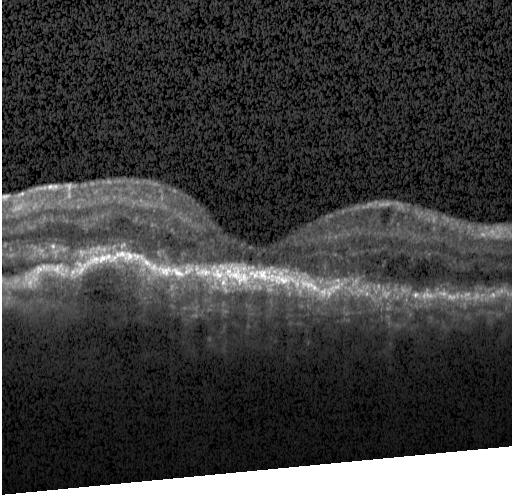

Horizontal scan through the fovea · spectral-domain OCT · retinal OCT B-scan · Heidelberg Spectralis — Impression: choroidal neovascularization (CNV).